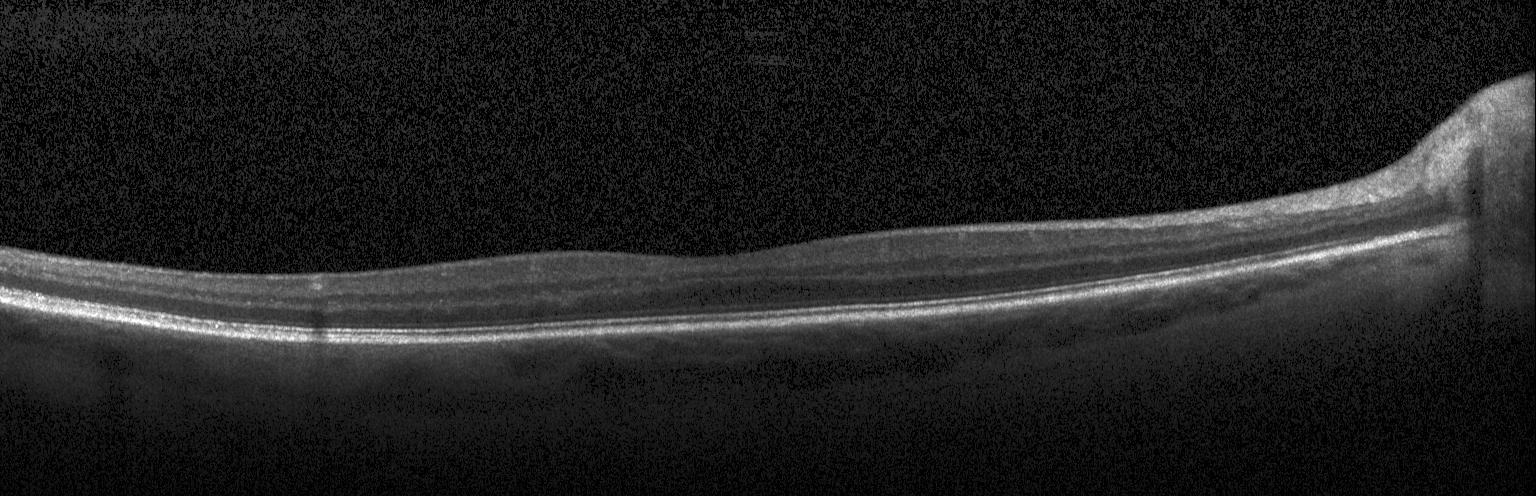

Instrument: Heidelberg Spectralis. Retinal OCT cross-section. This B-scan demonstrates no evidence of CNV, DME, or drusen.